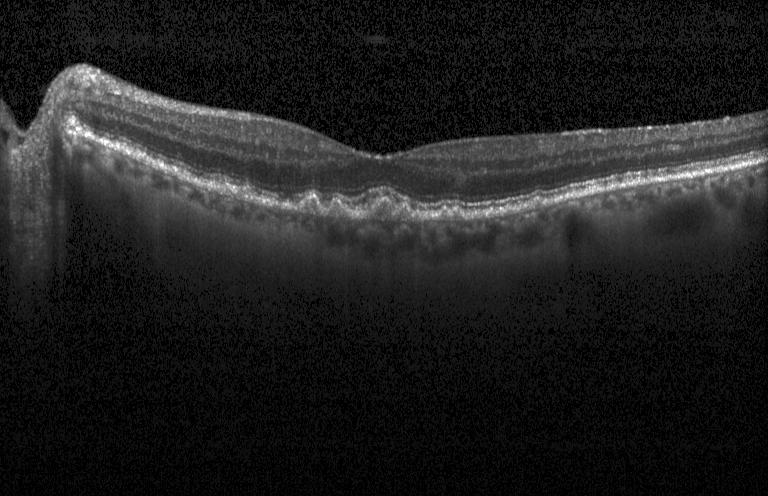

OCT finding: drusen.